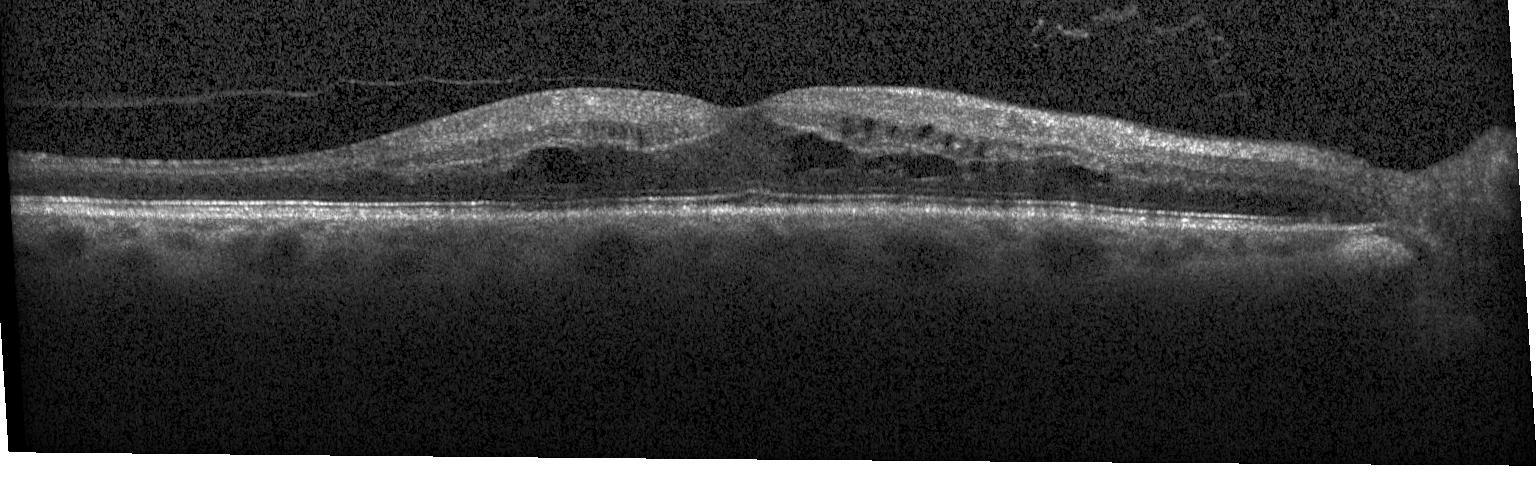 OCT scan showing diabetic macular edema.